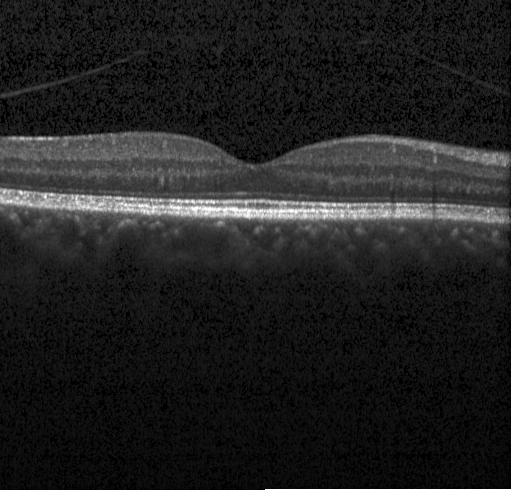
Acquired on a Heidelberg Spectralis. Optical coherence tomography B-scan. Macular scan. Macular OCT: no choroidal neovascularization, no diabetic macular edema, and no drusen.